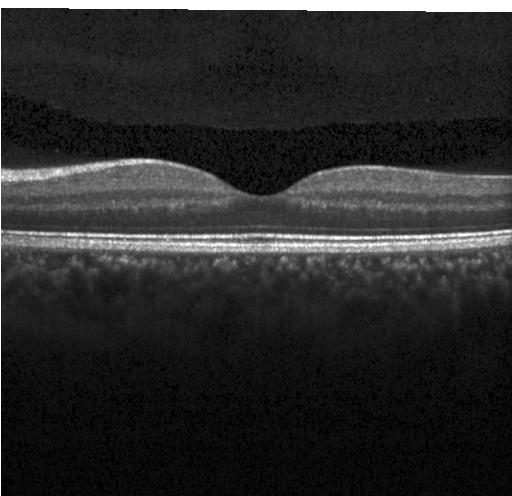
Instrument: Heidelberg Spectralis, SD-OCT, OCT line scan.
Assessment: no evidence of choroidal neovascularization, diabetic macular edema, or drusen.